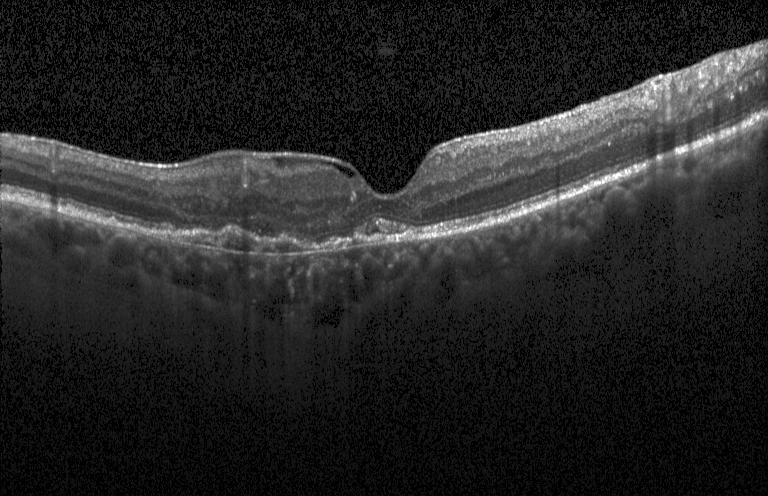 OCT B-scan; through the macula; spectral-domain optical coherence tomography. Impression: a choroidal neovascular membrane.